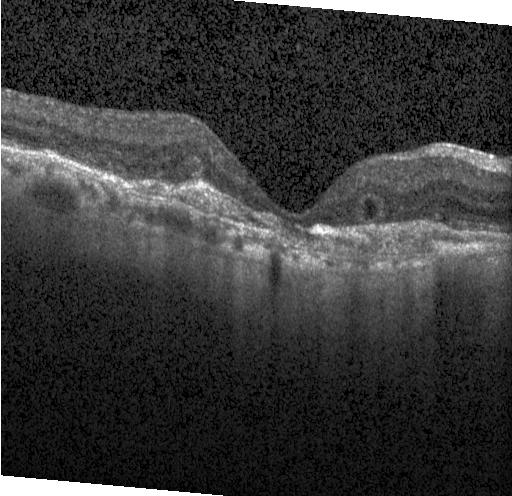

Finding: choroidal neovascularization.